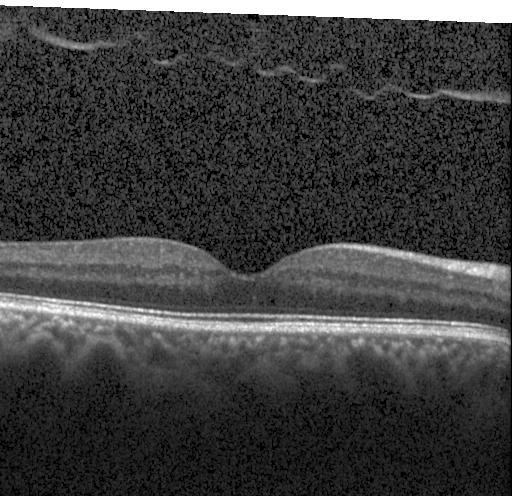
Horizontal scan through the fovea; optical coherence tomography B-scan. Macular OCT: neither CNV, DME, nor drusen.